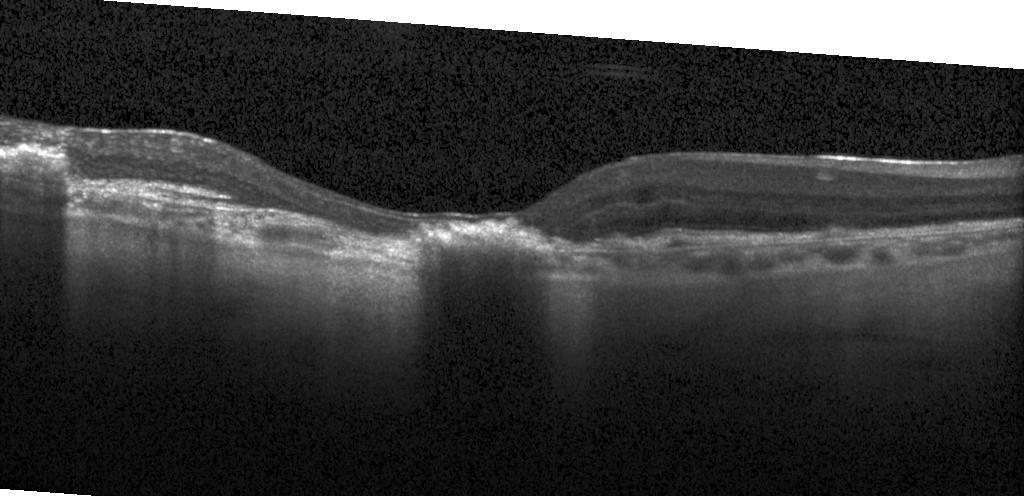
OCT B-scan. Diagnosis: a choroidal neovascular membrane.